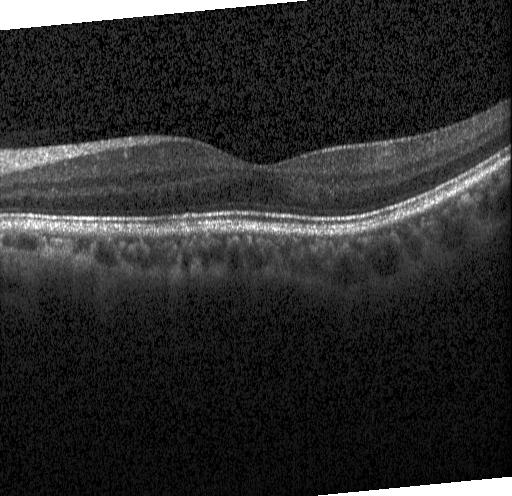

Through the macula · acquired on a Heidelberg Spectralis · OCT B-scan. Finding: no CNV, no DME, and no drusen.